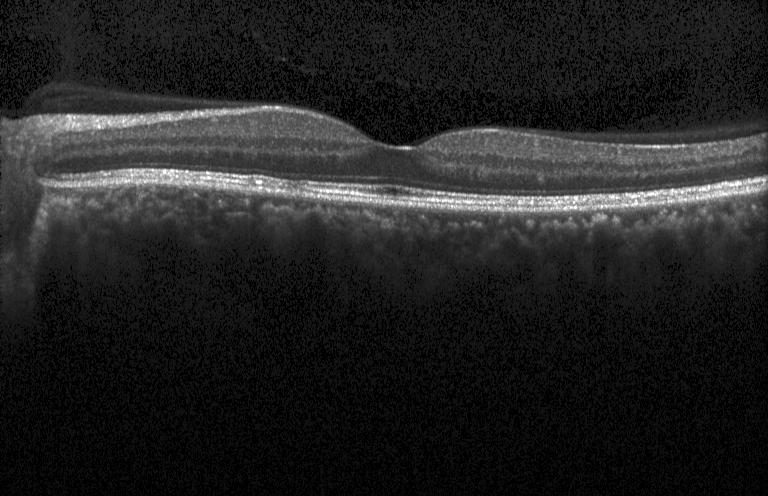

Optical coherence tomography B-scan, macular scan, SD-OCT, acquired on a Heidelberg Spectralis. Dx: neither CNV, DME, nor drusen.